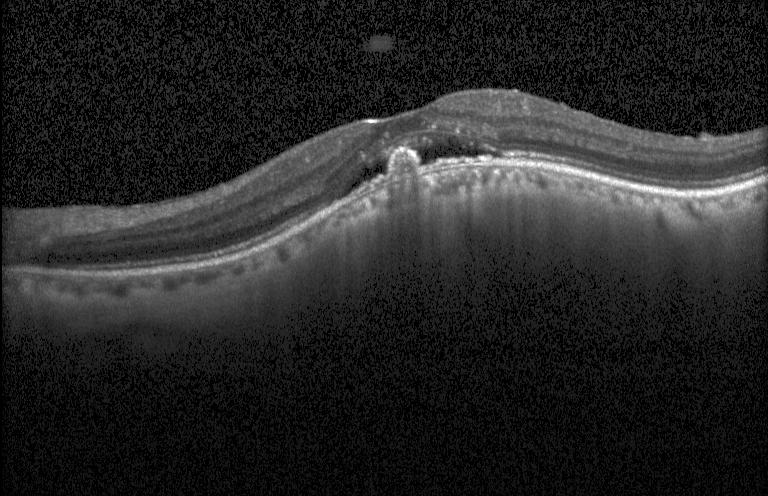 Optical coherence tomography B-scan. Horizontal scan through the fovea. SD-OCT. Heidelberg Spectralis OCT system.
Finding: a choroidal neovascular membrane.